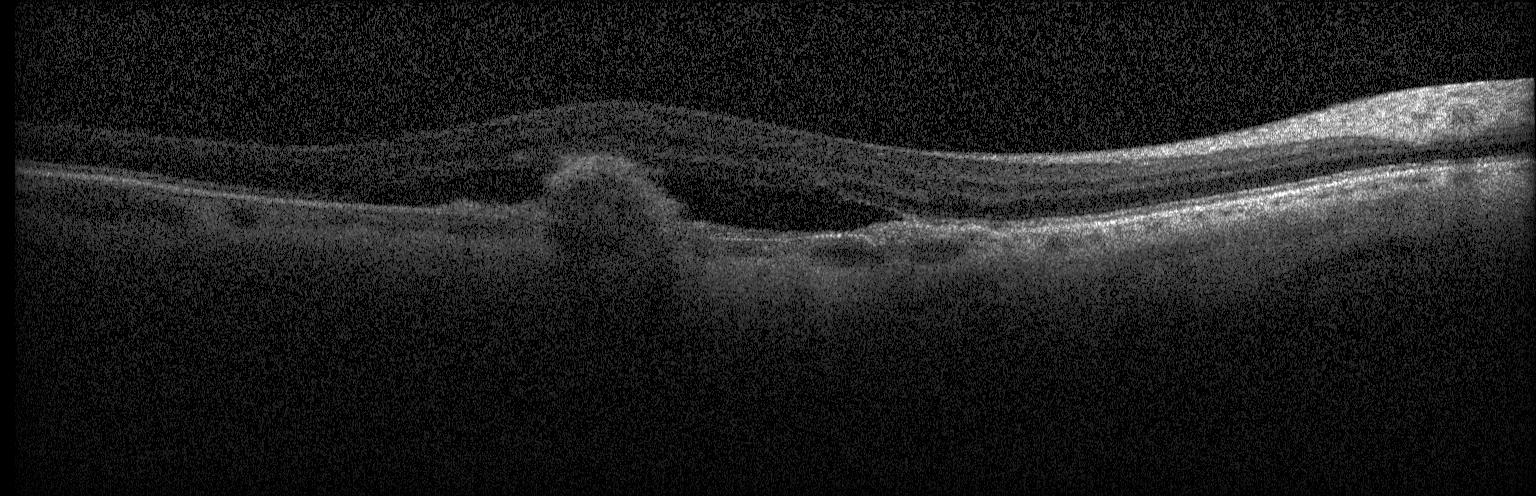

Fovea-centered; spectral-domain optical coherence tomography; retinal OCT cross-section.
Diagnosis: choroidal neovascularization (CNV).